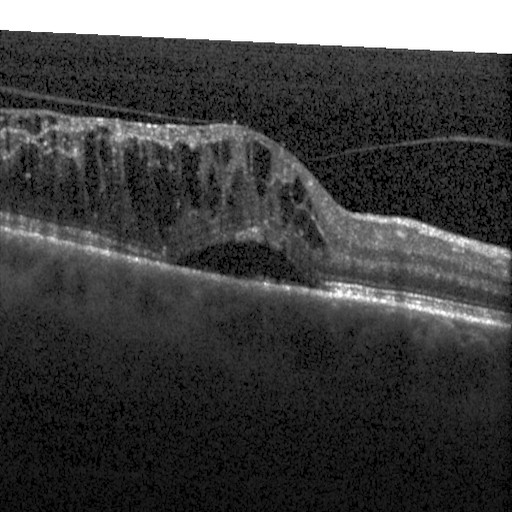

Diagnosis: DME.